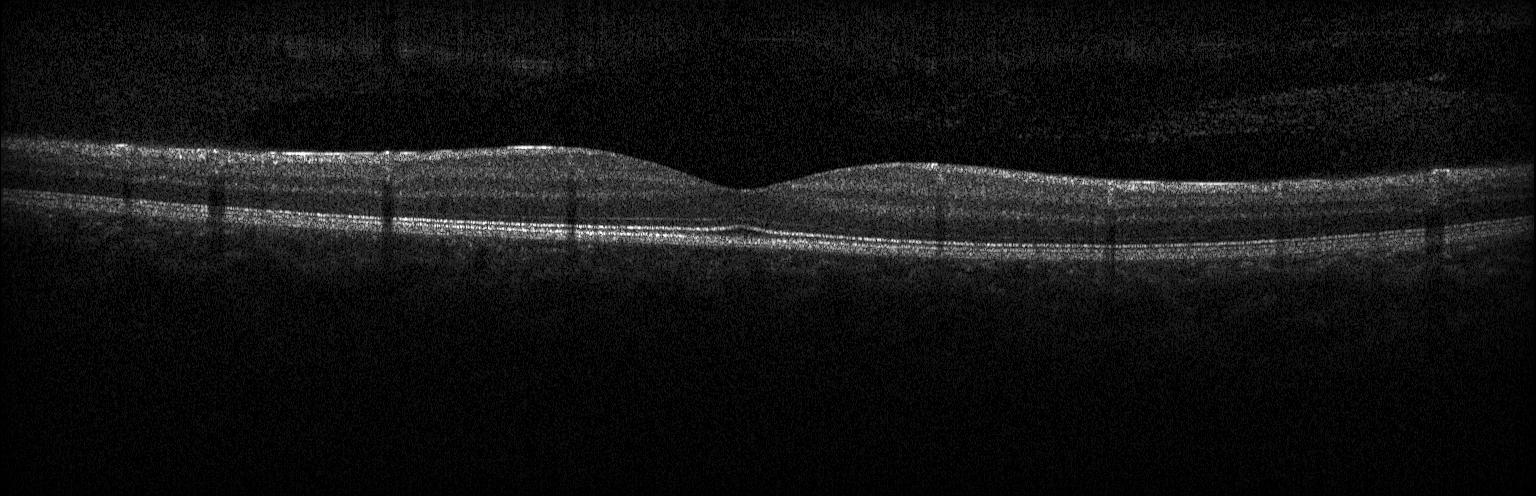 Optical coherence tomography B-scan. No evidence of choroidal neovascularization, diabetic macular edema, or drusen.